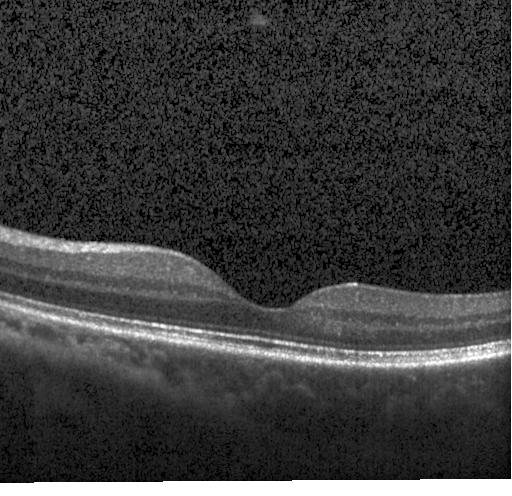 Diagnosis: no CNV, no DME, and no drusen.